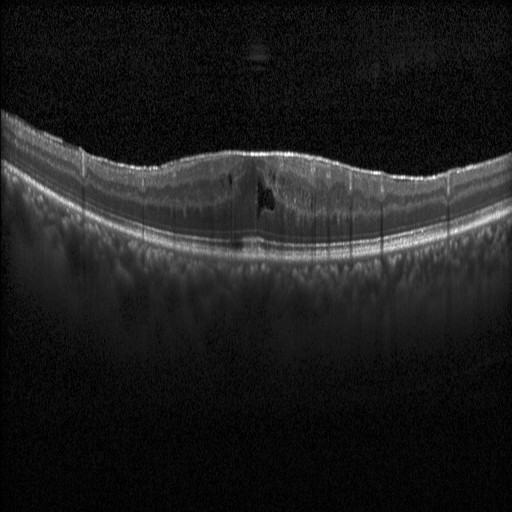
SD-OCT · OCT B-scan. Diabetic macular edema (DME).